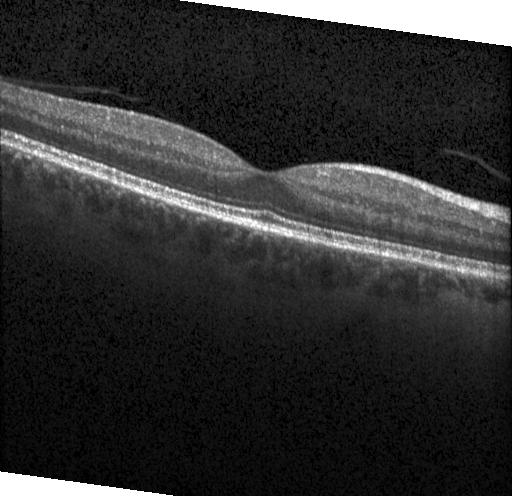
Fovea-centered; instrument: Heidelberg Spectralis; optical coherence tomography B-scan; spectral-domain OCT — No CNV, no DME, and no drusen.